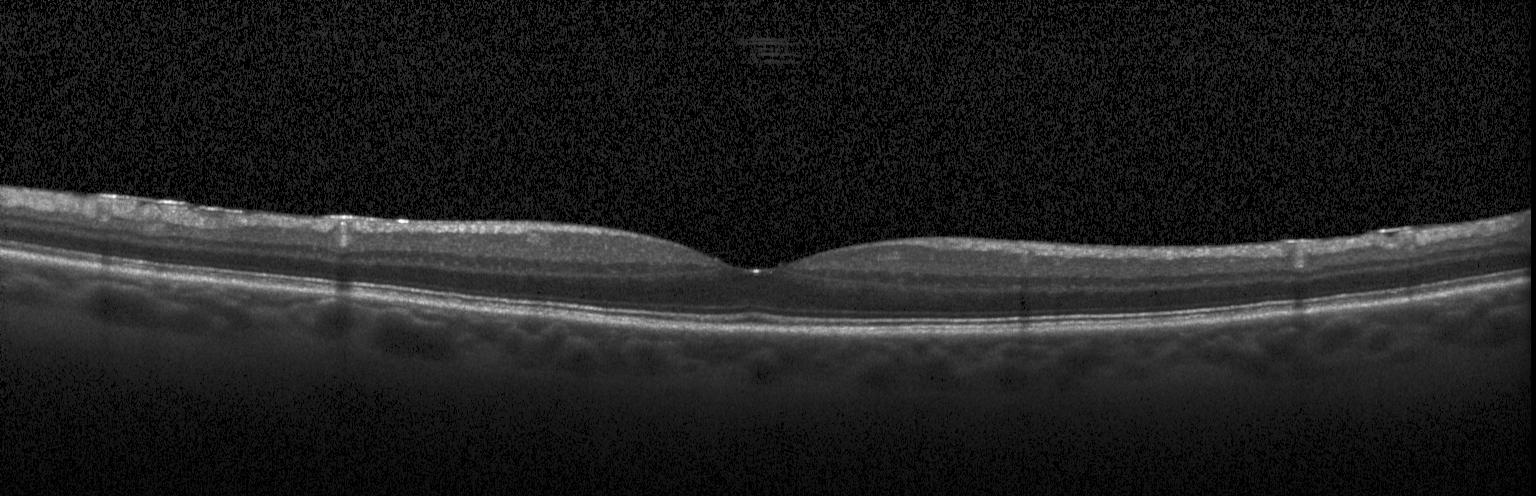
Spectral-domain OCT B-scan: no evidence of choroidal neovascularization, diabetic macular edema, or drusen.